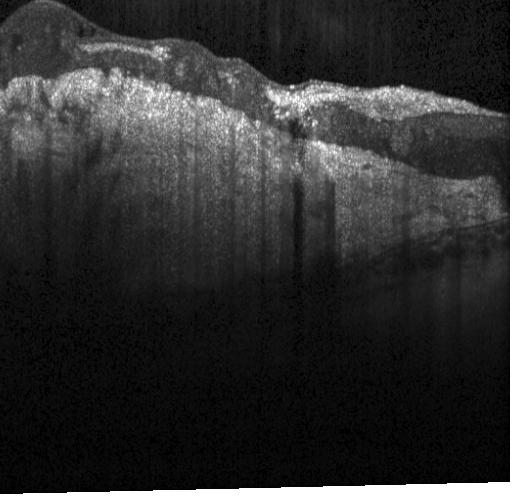

Fovea-centered; Heidelberg Spectralis OCT system; optical coherence tomography scan
Impression: CNV.